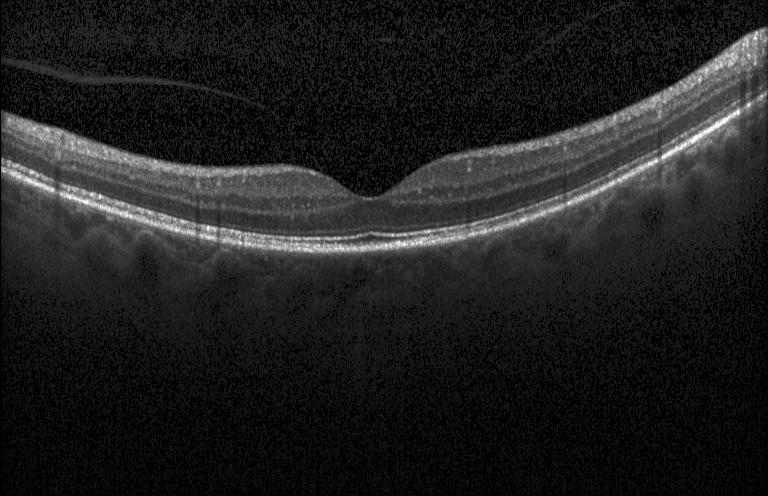
Heidelberg Spectralis OCT system, retinal OCT cross-section.
Macular OCT: neither CNV, DME, nor drusen.